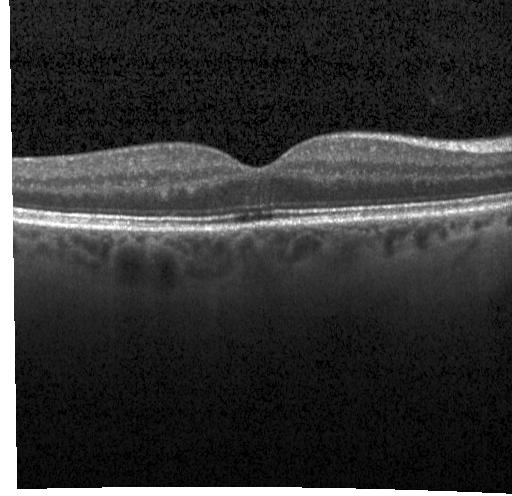 Finding: no choroidal neovascularization, diabetic macular edema, or drusen.